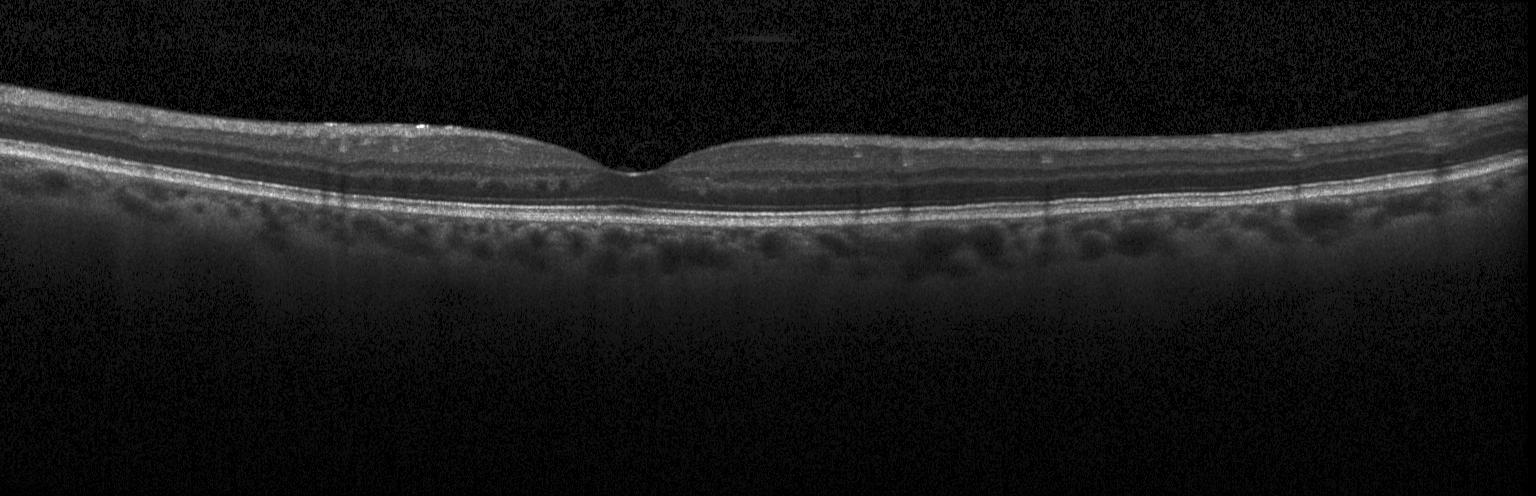
Optical coherence tomography B-scan
The scan shows no evidence of choroidal neovascularization, diabetic macular edema, or drusen.